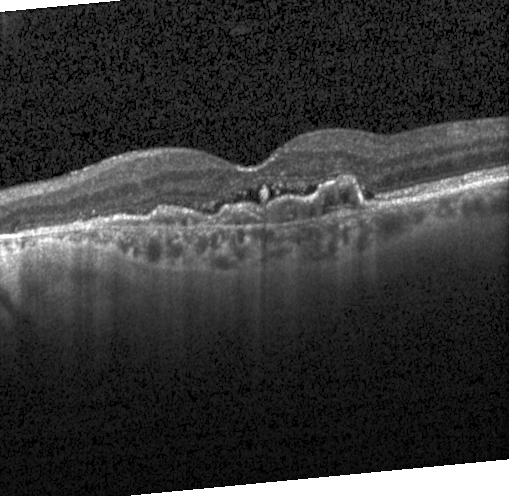
A choroidal neovascular membrane.